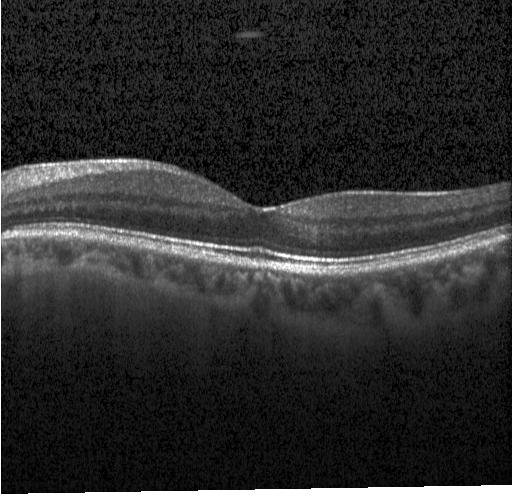

Finding: neither choroidal neovascularization, diabetic macular edema, nor drusen.